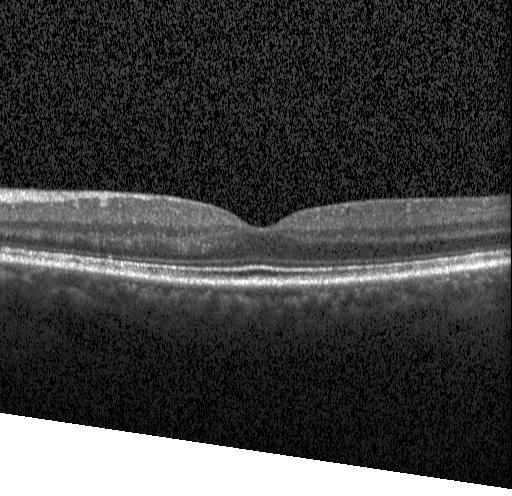
OCT B-scan showing no CNV, DME, or drusen.